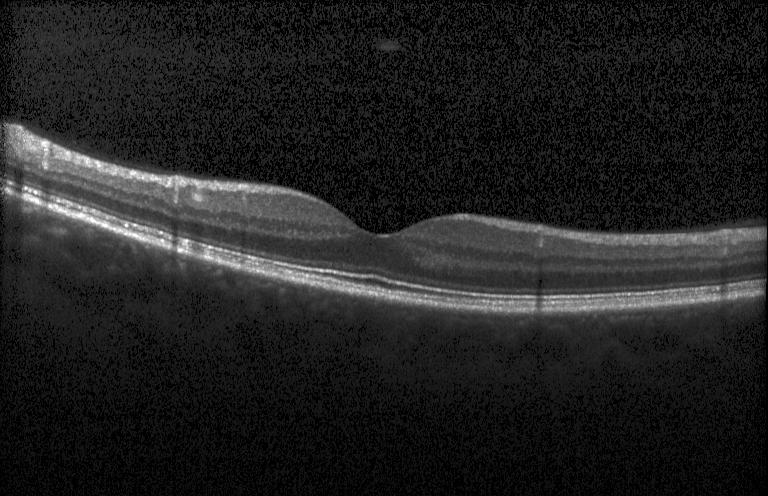 SD-OCT, instrument: Heidelberg Spectralis, OCT B-scan — Finding: no choroidal neovascularization, no diabetic macular edema, and no drusen.